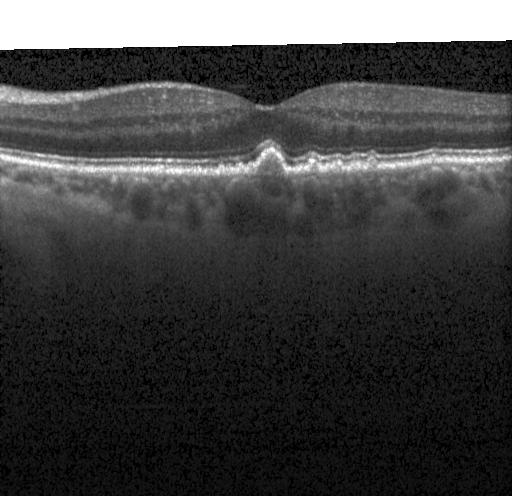

Centered on the fovea, Heidelberg Spectralis OCT system, OCT B-scan
Finding: multiple drusen.